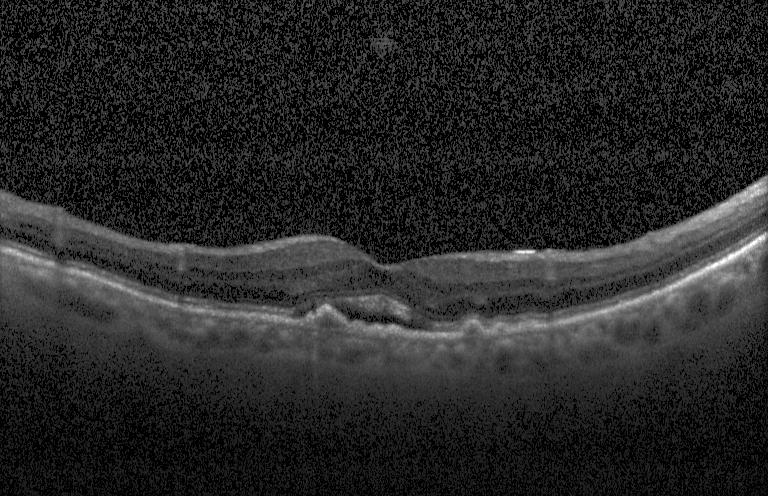

Finding: choroidal neovascularization.